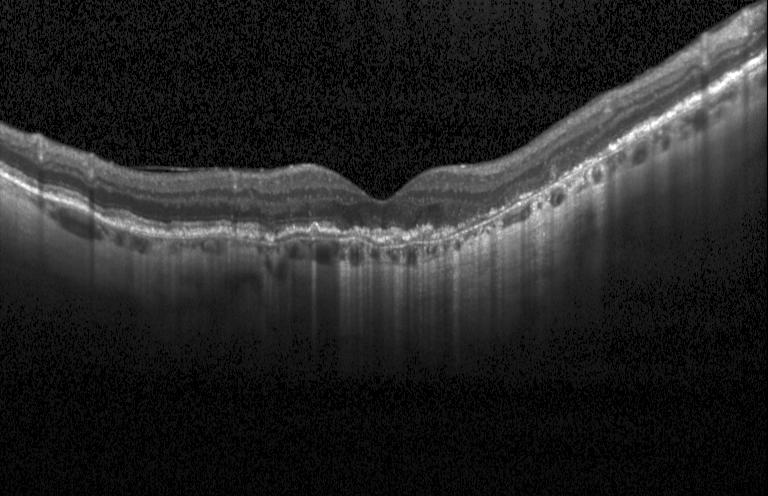

Finding: a choroidal neovascular membrane.